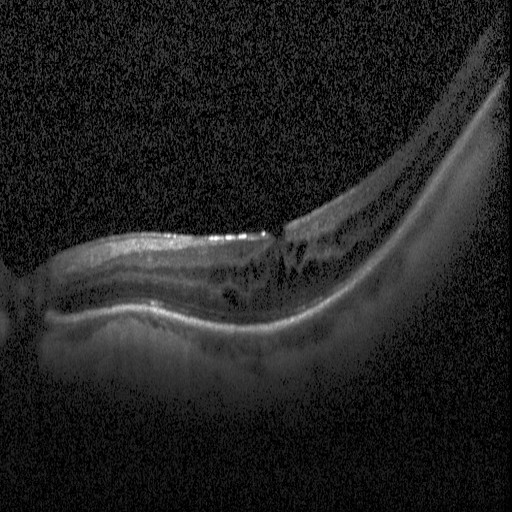
OCT finding: DME.